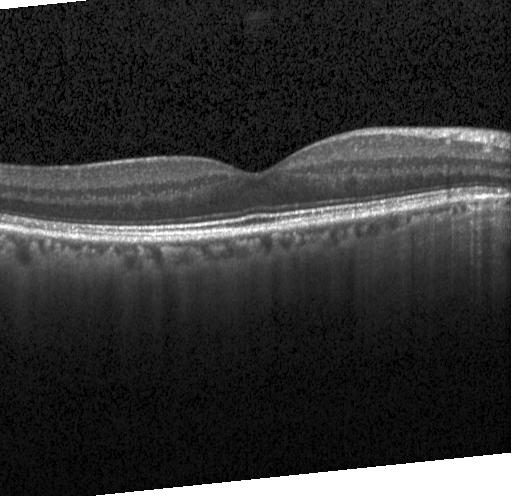
OCT line scan. No CNV, DME, or drusen.